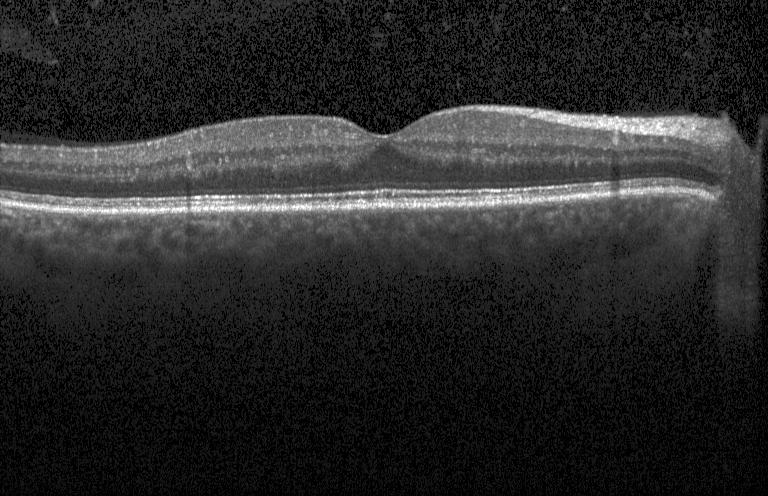
Optical coherence tomography scan. Assessment: no choroidal neovascularization, no diabetic macular edema, and no drusen.